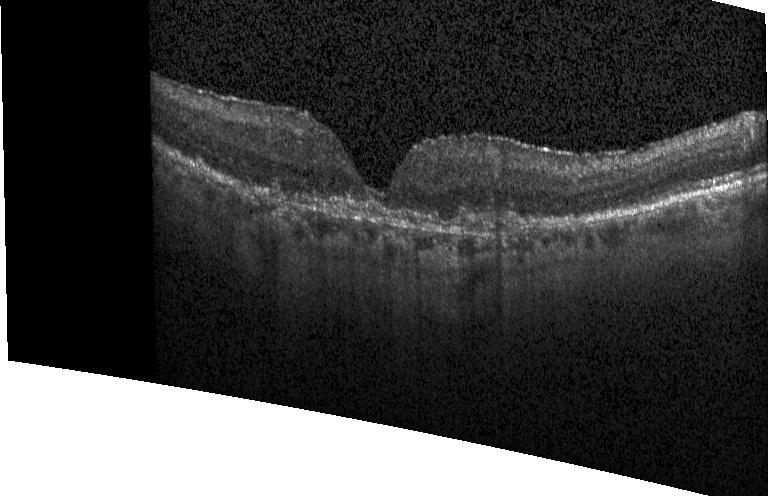 Centered on the fovea. Optical coherence tomography B-scan
Impression: a choroidal neovascular membrane.